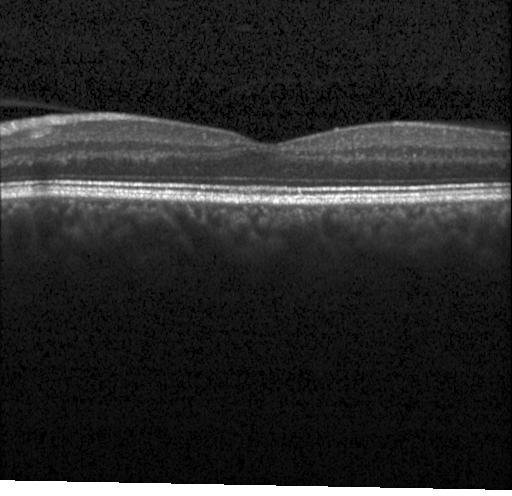 Spectral-domain OCT B-scan: neither CNV, DME, nor drusen.